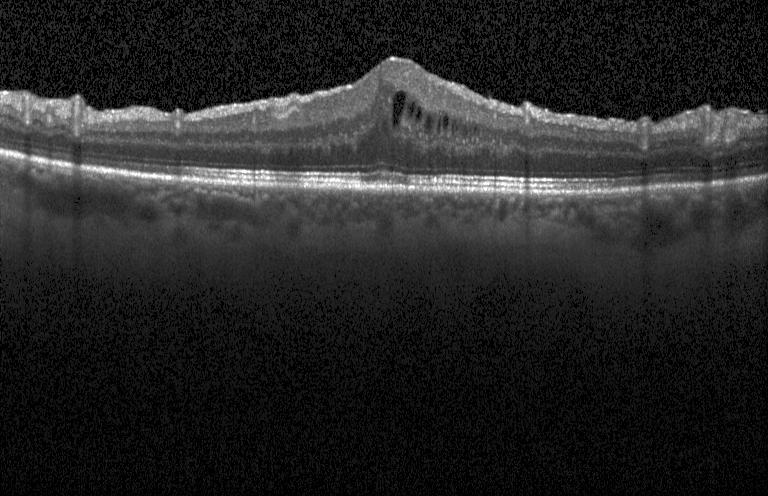
Macular OCT: diabetic macular edema (DME).